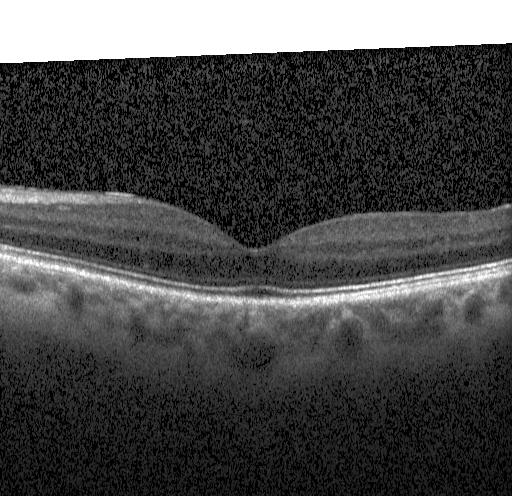
Horizontal scan through the fovea; Heidelberg Spectralis; retinal OCT B-scan; spectral-domain optical coherence tomography.
Finding: no evidence of choroidal neovascularization, diabetic macular edema, or drusen.